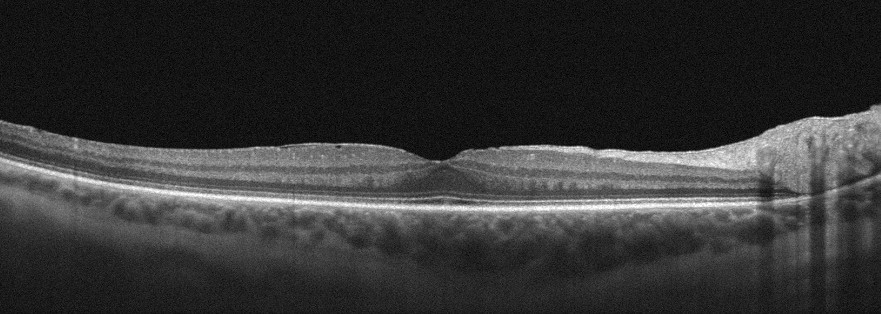

Fovea-centered; retinal OCT cross-section. Diagnosis: ERM.